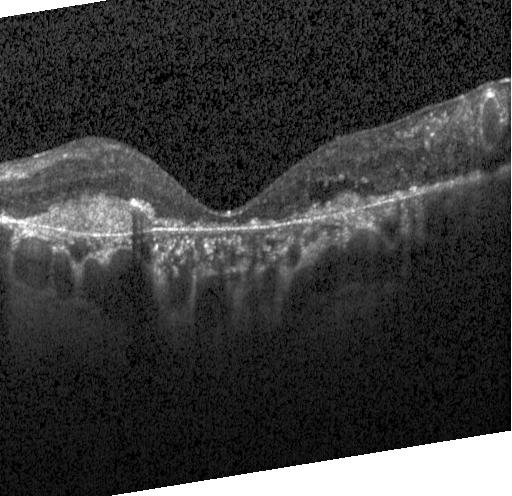 Retinal OCT cross-section showing a choroidal neovascular membrane.